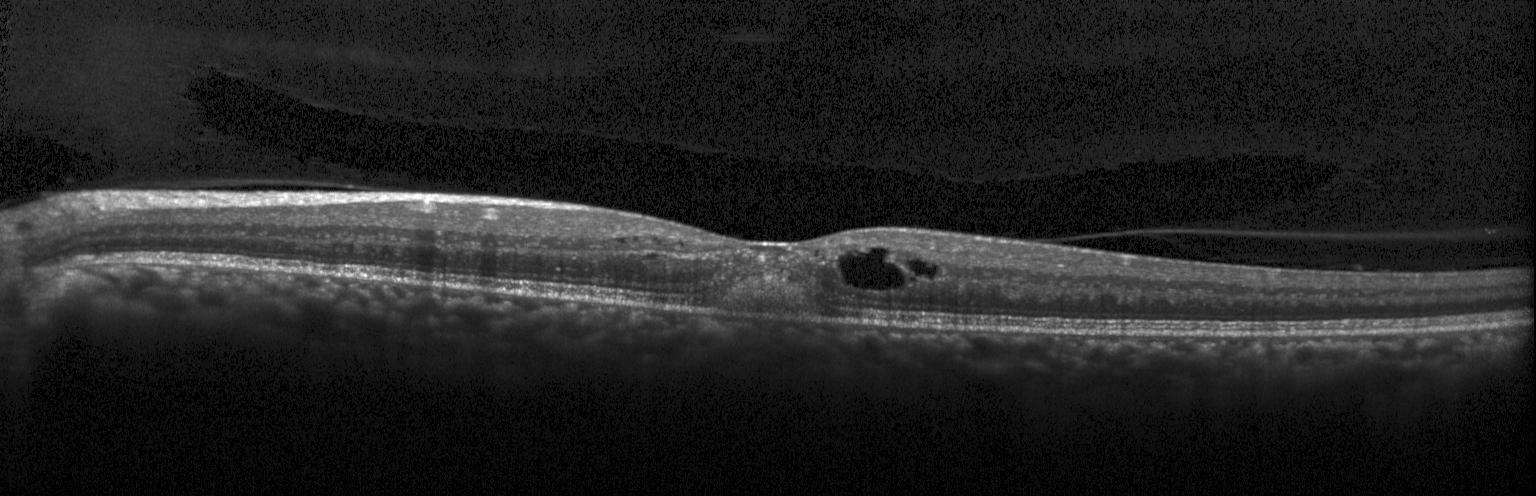 Retinal OCT B-scan — Dx: a choroidal neovascular membrane.